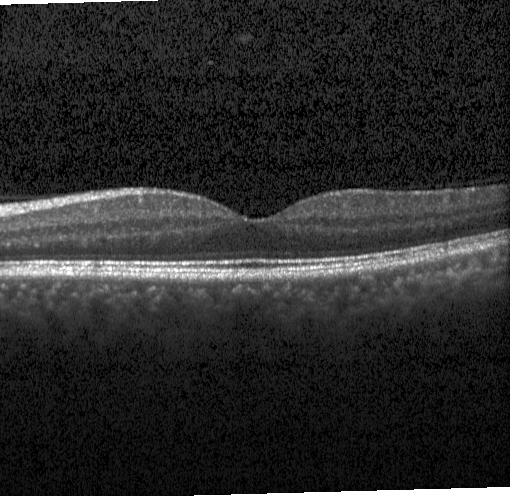 Fovea-centered, retinal OCT B-scan. Diagnosis: neither CNV, DME, nor drusen.